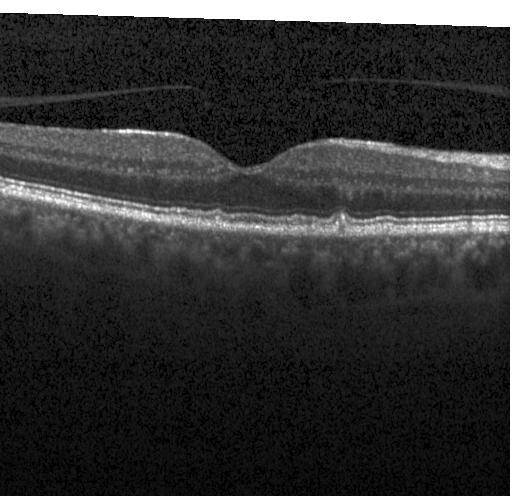
Dx: drusen.